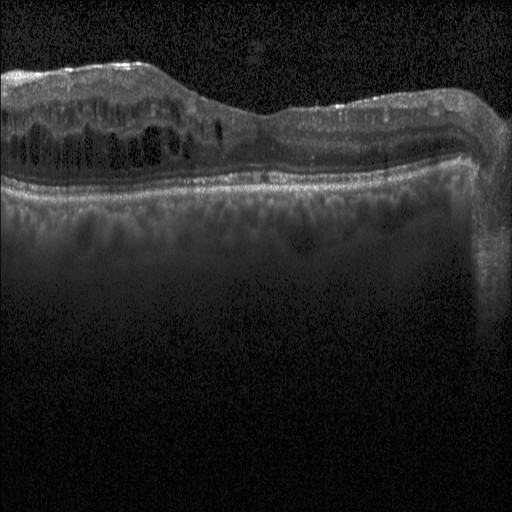

Optical coherence tomography scan; horizontal scan through the fovea — This B-scan demonstrates diabetic macular edema.